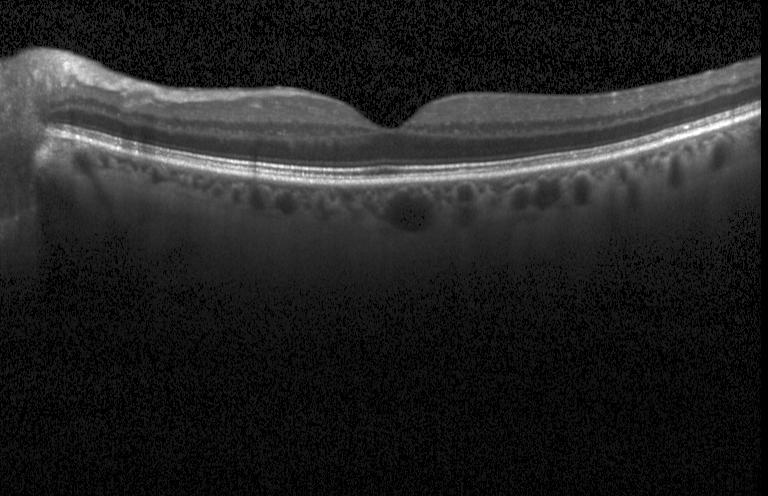

Optical coherence tomography B-scan. Acquired on a Heidelberg Spectralis. Horizontal scan through the fovea. This B-scan demonstrates no evidence of choroidal neovascularization, diabetic macular edema, or drusen.